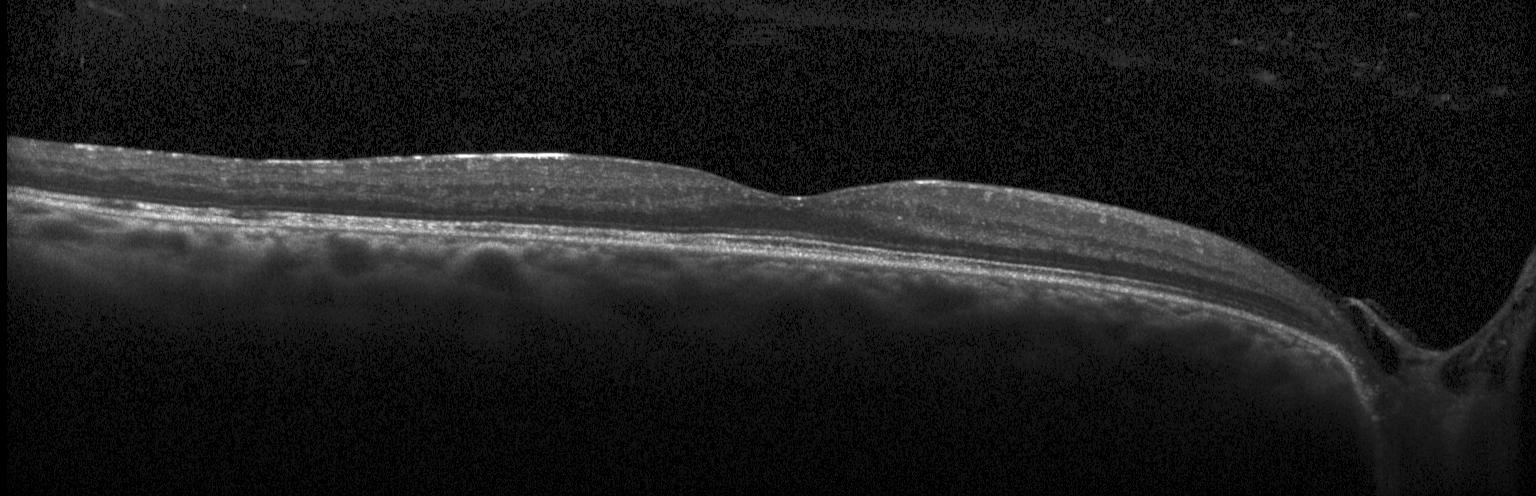 No evidence of choroidal neovascularization, diabetic macular edema, or drusen.